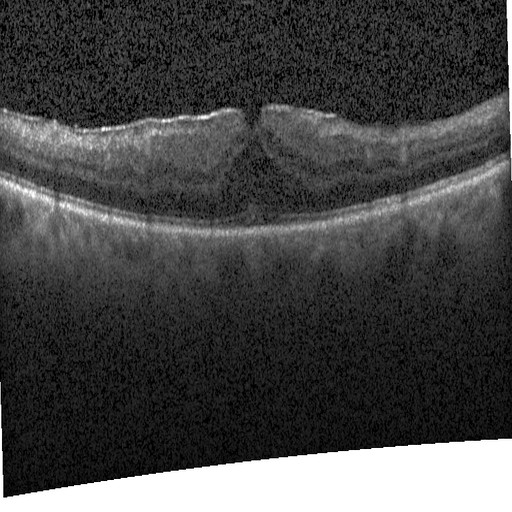
Horizontal scan through the fovea; optical coherence tomography scan; Heidelberg Spectralis OCT system; spectral-domain optical coherence tomography. Diagnosis: DME.